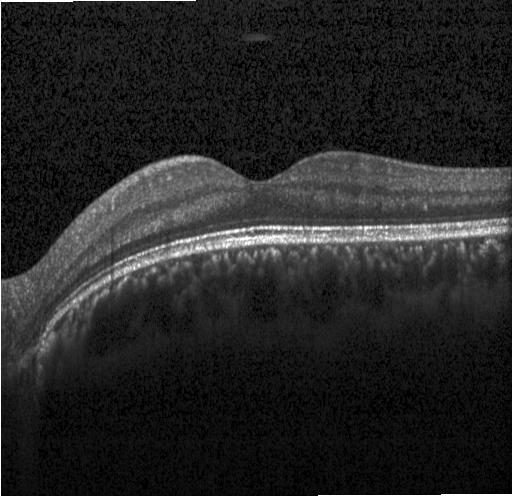 Diagnosis: no choroidal neovascularization, diabetic macular edema, or drusen.